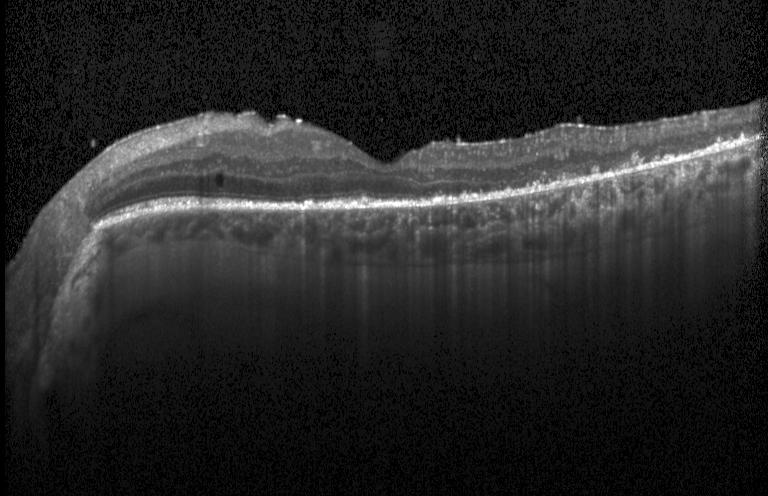 OCT B-scan. Spectral-domain OCT. Horizontal scan through the fovea. Heidelberg Spectralis OCT system
Finding: diabetic macular edema (DME).